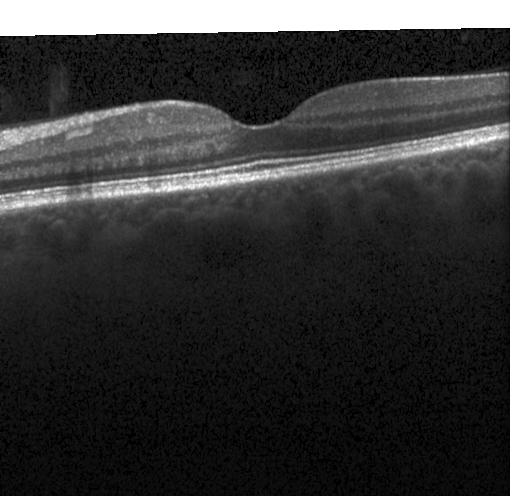
Macular OCT: no evidence of choroidal neovascularization, diabetic macular edema, or drusen.